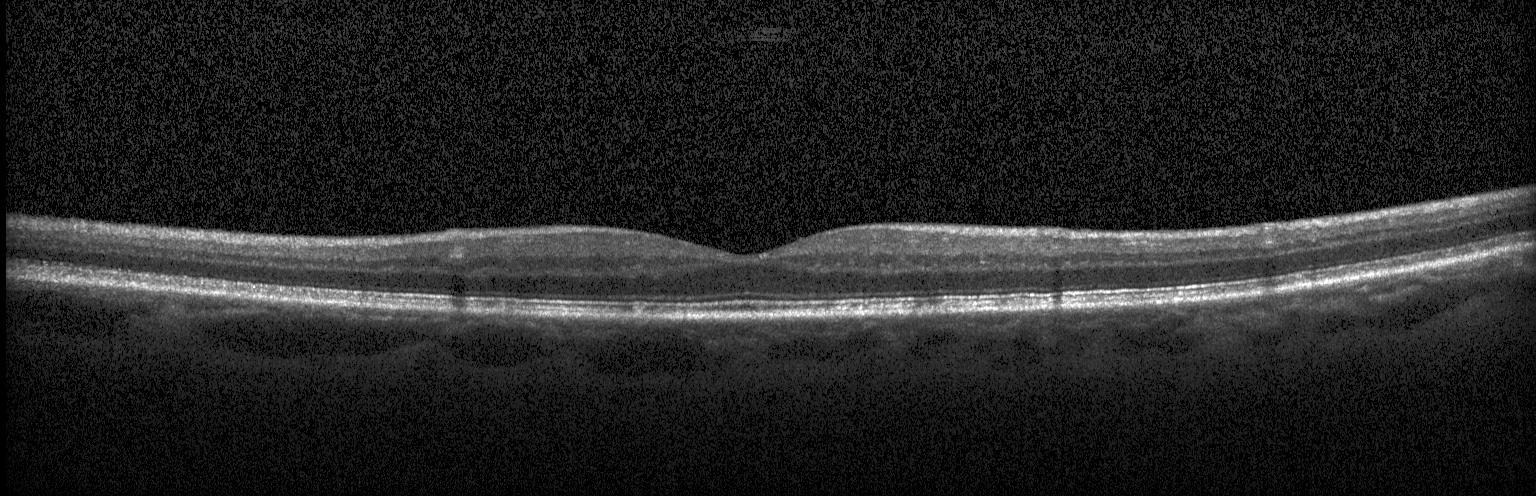

OCT B-scan. Horizontal scan through the fovea
Finding: no choroidal neovascularization, no diabetic macular edema, and no drusen.